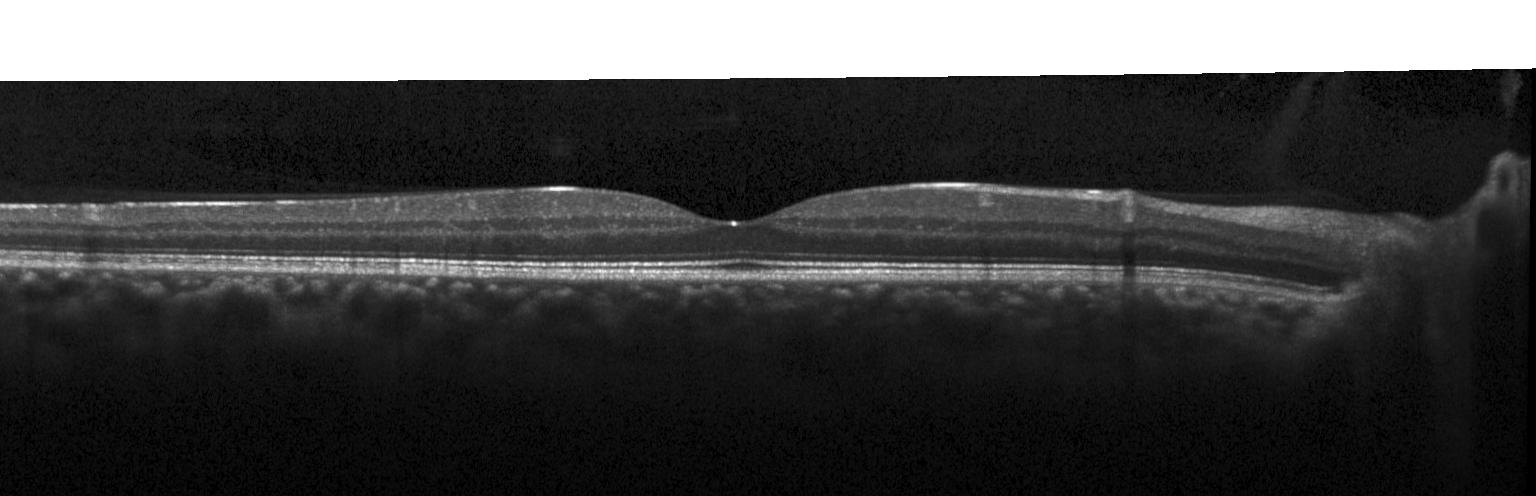

Retinal OCT cross-section. Diagnosis: no choroidal neovascularization, no diabetic macular edema, and no drusen.